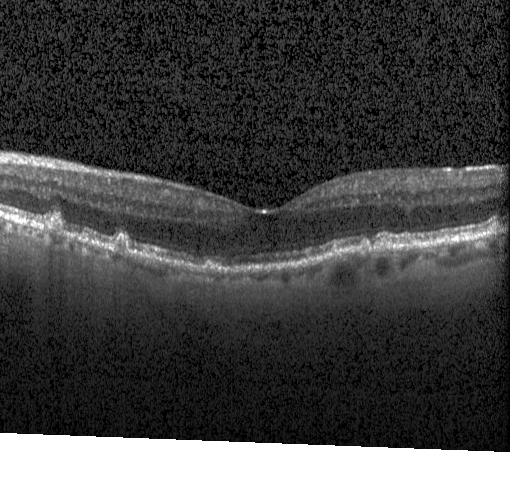 Spectral-domain OCT. Retinal OCT B-scan. Macular scan. Instrument: Heidelberg Spectralis.
Drusen.